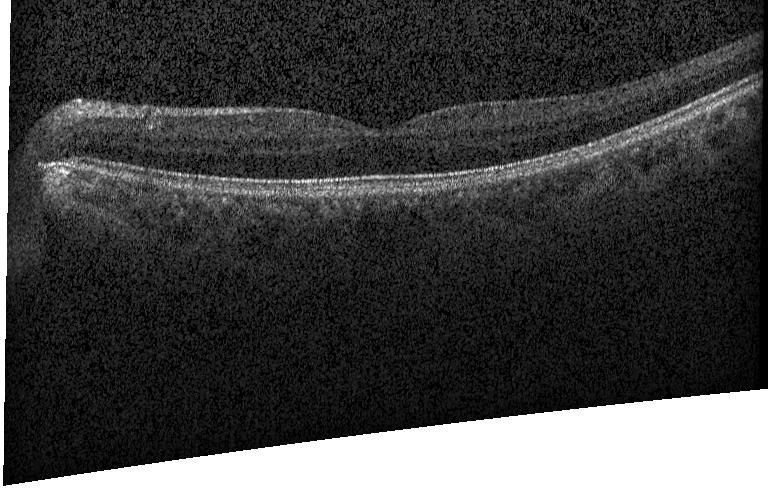
Retinal OCT cross-section; instrument: Heidelberg Spectralis; fovea-centered
Diagnosis: no evidence of choroidal neovascularization, diabetic macular edema, or drusen.